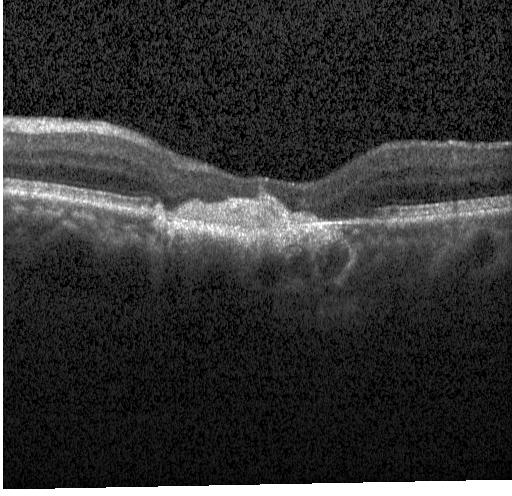 Finding: a choroidal neovascular membrane.